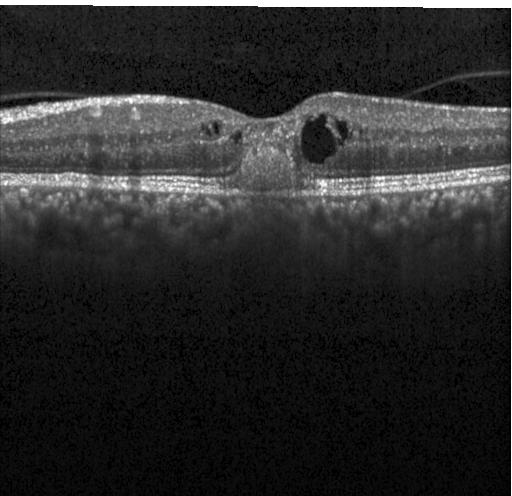
OCT B-scan; acquired on a Heidelberg Spectralis.
Dx: a choroidal neovascular membrane.